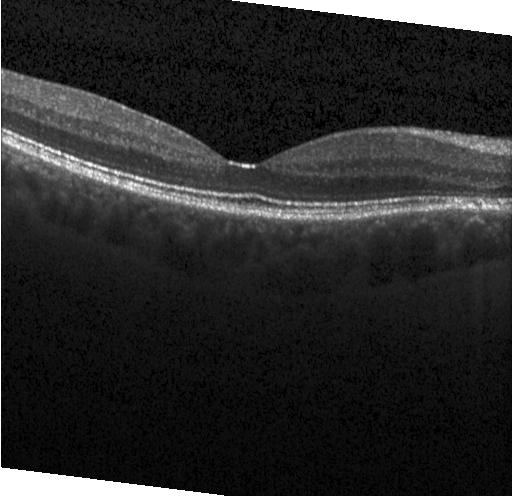
Fovea-centered · OCT B-scan. Finding: no choroidal neovascularization, diabetic macular edema, or drusen.